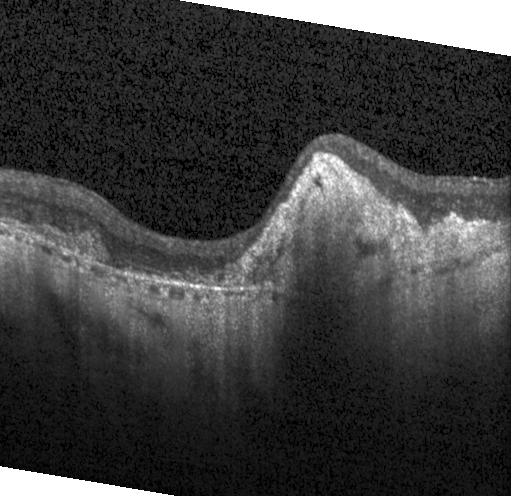 OCT B-scan showing a choroidal neovascular membrane.